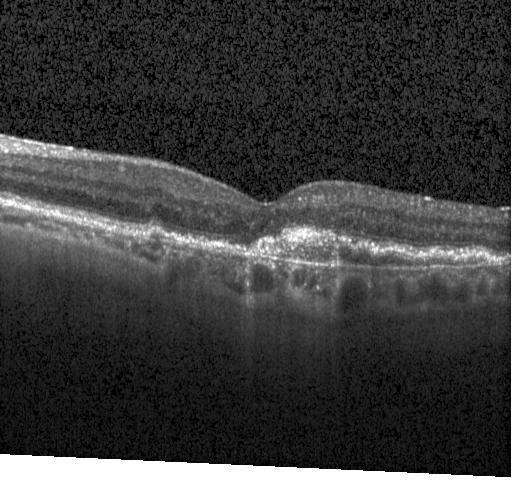 Through the macula; optical coherence tomography B-scan; spectral-domain OCT; Heidelberg Spectralis. Finding: a choroidal neovascular membrane.